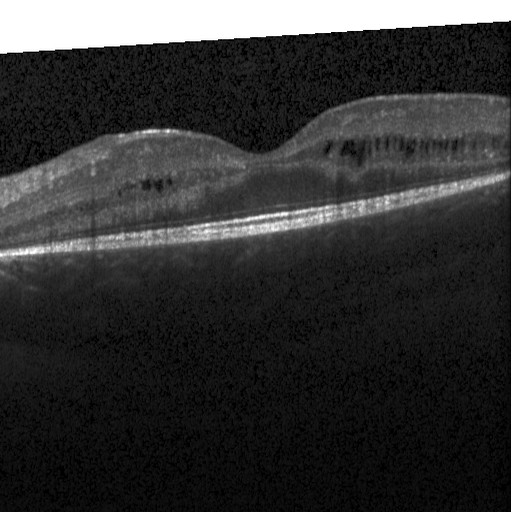 Instrument: Heidelberg Spectralis; optical coherence tomography scan
OCT finding: diabetic macular edema.